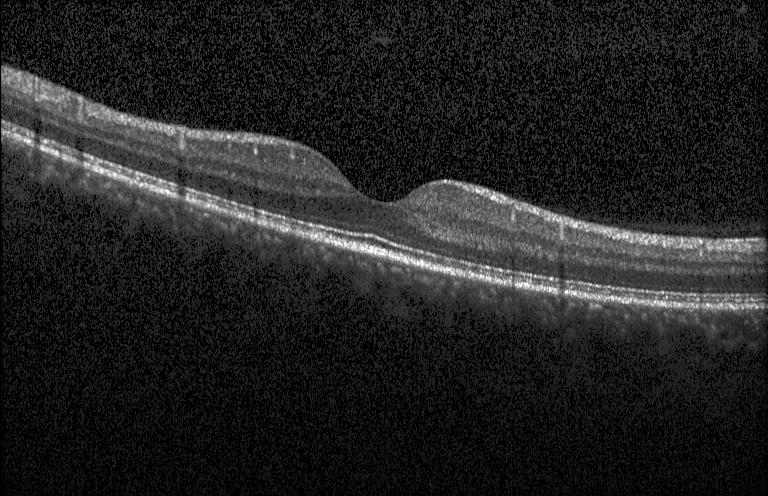
Optical coherence tomography scan · spectral-domain optical coherence tomography — Impression: no choroidal neovascularization, no diabetic macular edema, and no drusen.